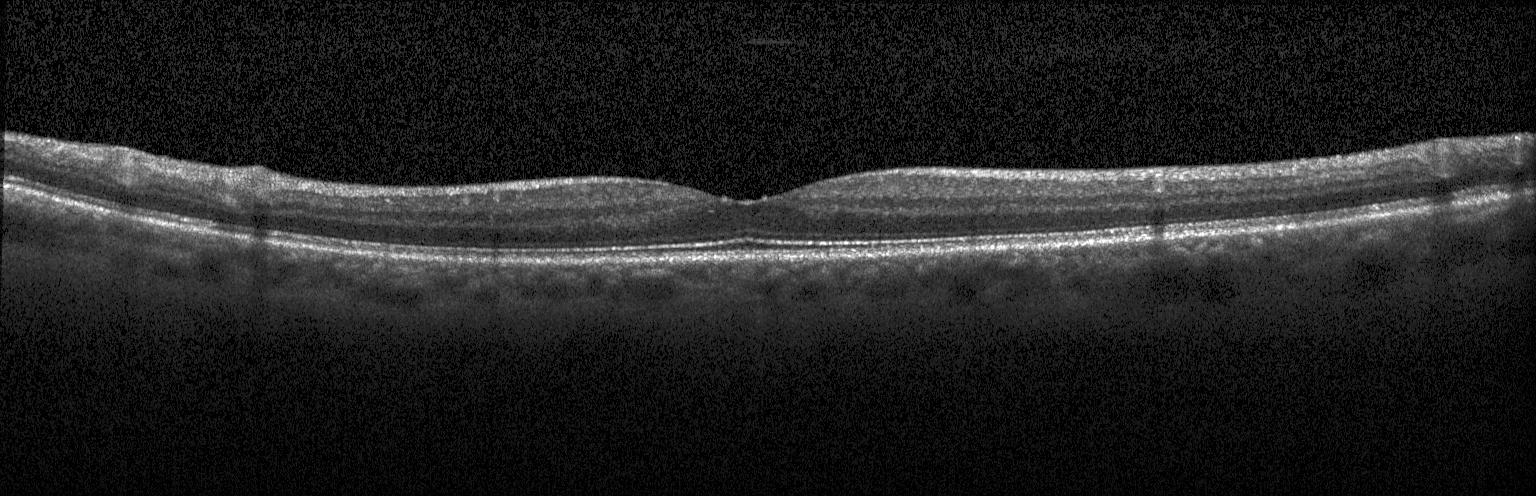
Macular scan, SD-OCT, optical coherence tomography B-scan — No choroidal neovascularization, no diabetic macular edema, and no drusen.